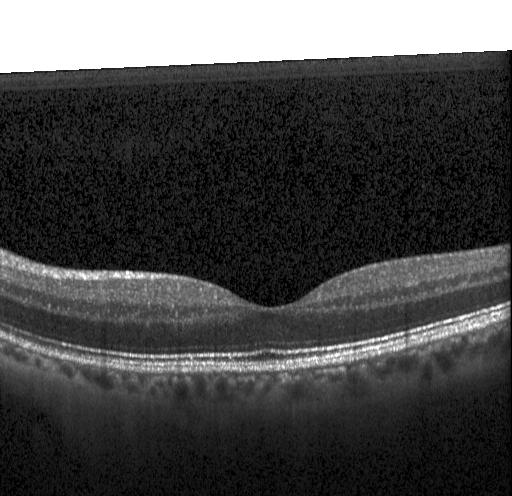

The scan shows no choroidal neovascularization, diabetic macular edema, or drusen.